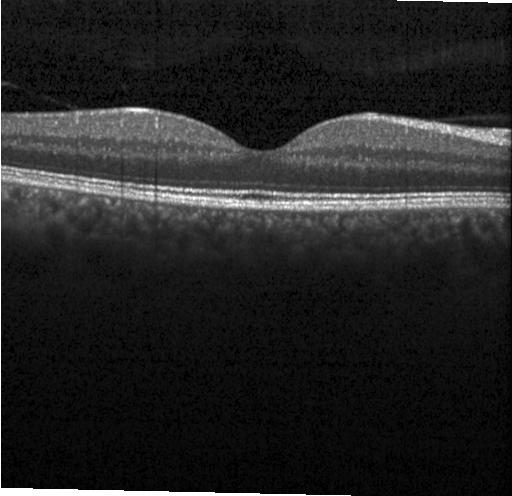

Optical coherence tomography scan
Impression: no evidence of choroidal neovascularization, diabetic macular edema, or drusen.